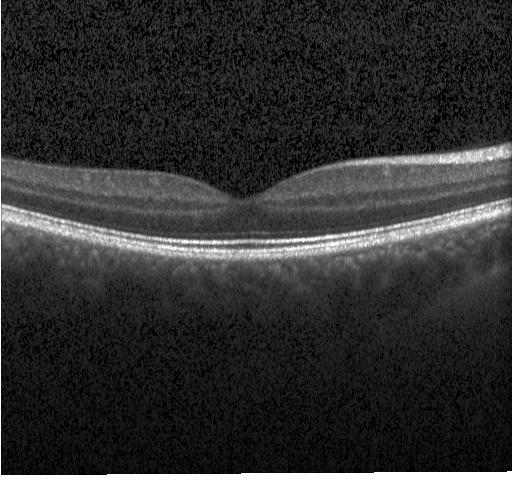

OCT line scan · Heidelberg Spectralis — The scan shows no CNV, no DME, and no drusen.